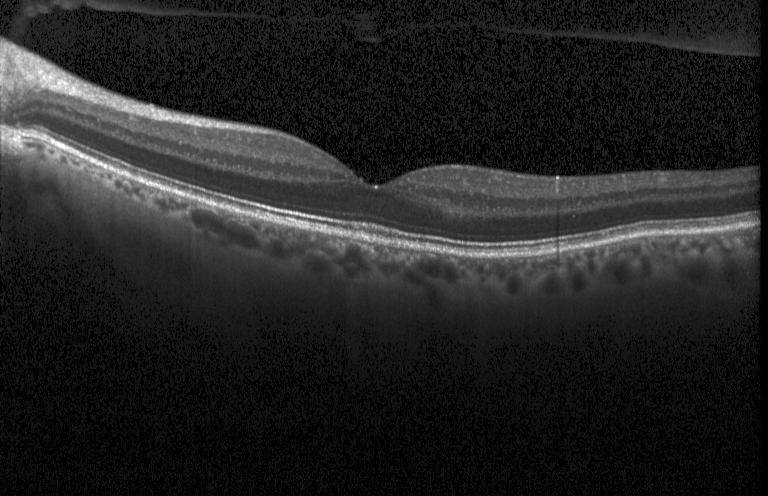 Assessment: no choroidal neovascularization, no diabetic macular edema, and no drusen.